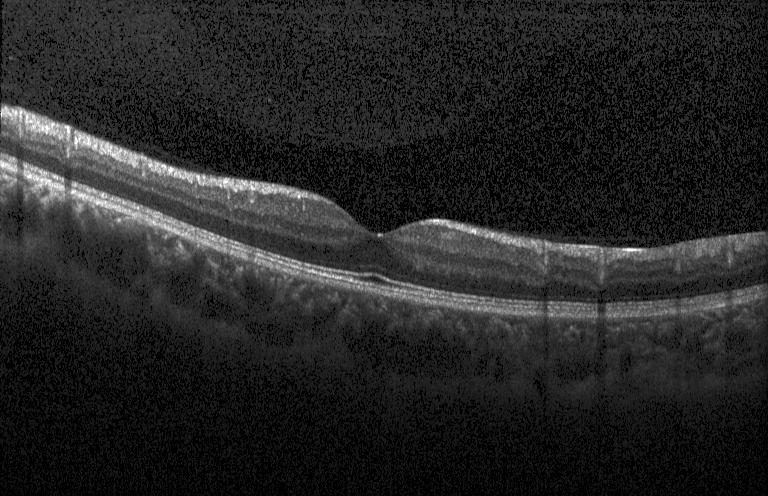 Spectral-domain OCT B-scan: no choroidal neovascularization, diabetic macular edema, or drusen.